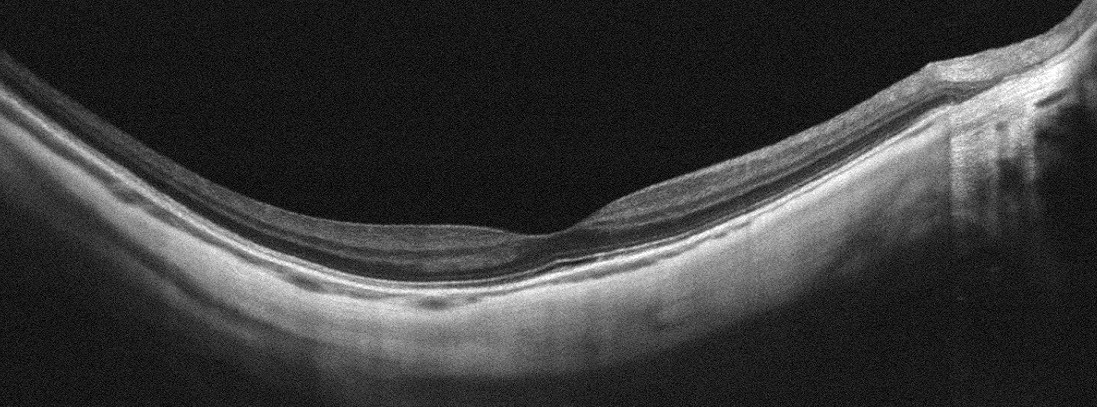 Finding: no evidence of AMD, DME, ERM, RAO, RVO, or VID.